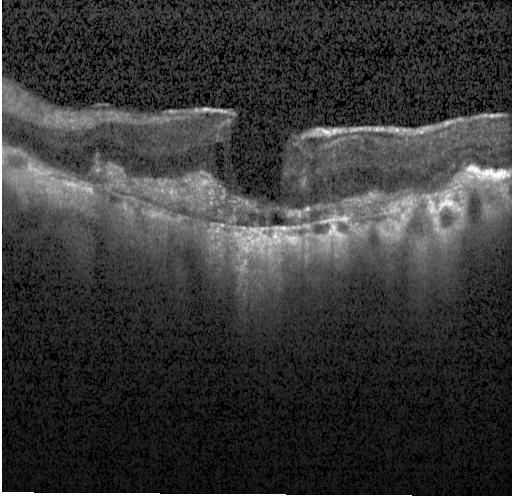 Horizontal scan through the fovea; optical coherence tomography scan. Dx: a choroidal neovascular membrane.